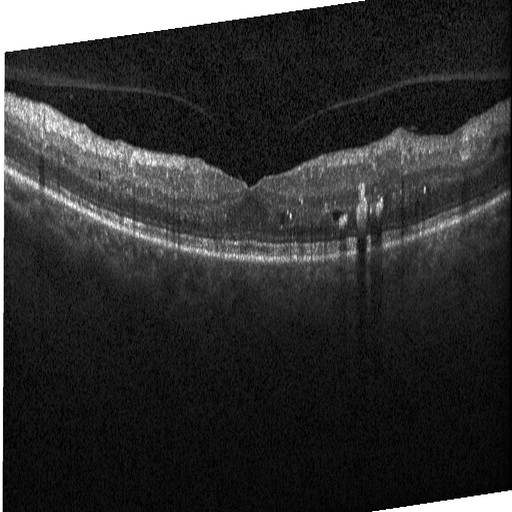
OCT B-scan · centered on the fovea · spectral-domain OCT · Heidelberg Spectralis
Assessment: DME.